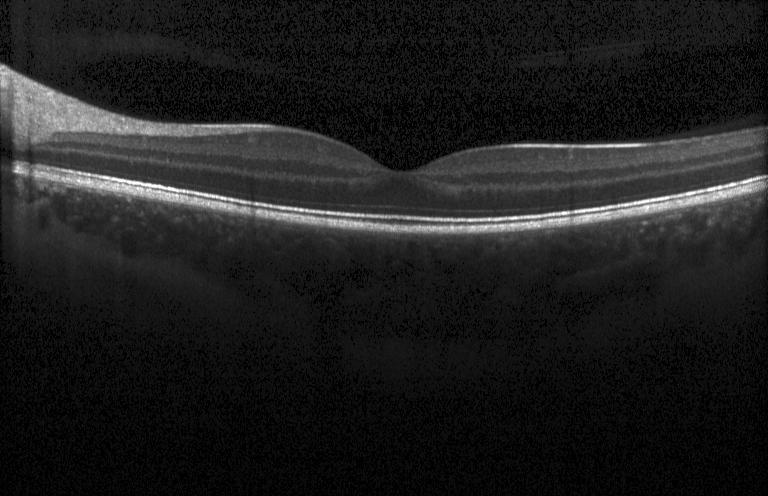 Spectral-domain optical coherence tomography. Horizontal scan through the fovea. Retinal OCT B-scan.
OCT finding: neither choroidal neovascularization, diabetic macular edema, nor drusen.